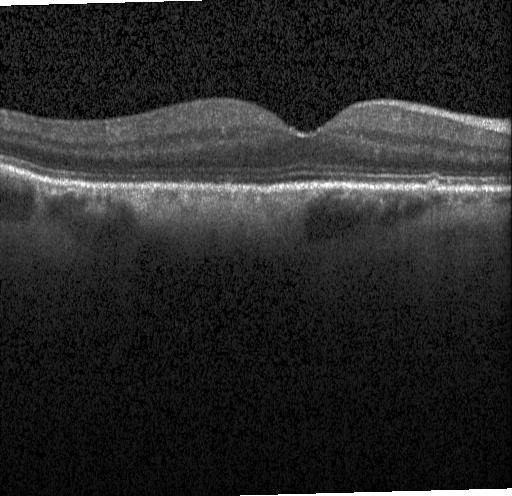

Diagnosis: drusen.